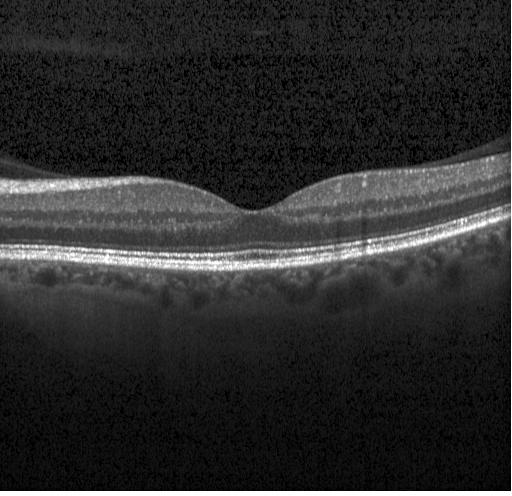 Spectral-domain OCT B-scan: neither CNV, DME, nor drusen.